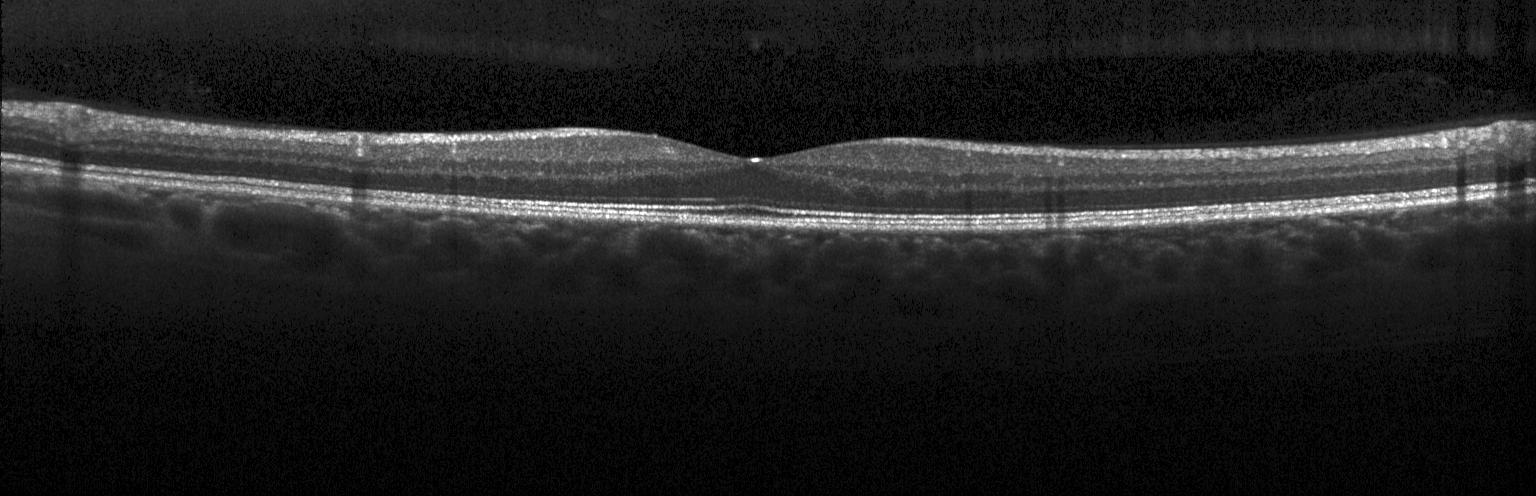
Finding: no choroidal neovascularization, diabetic macular edema, or drusen.